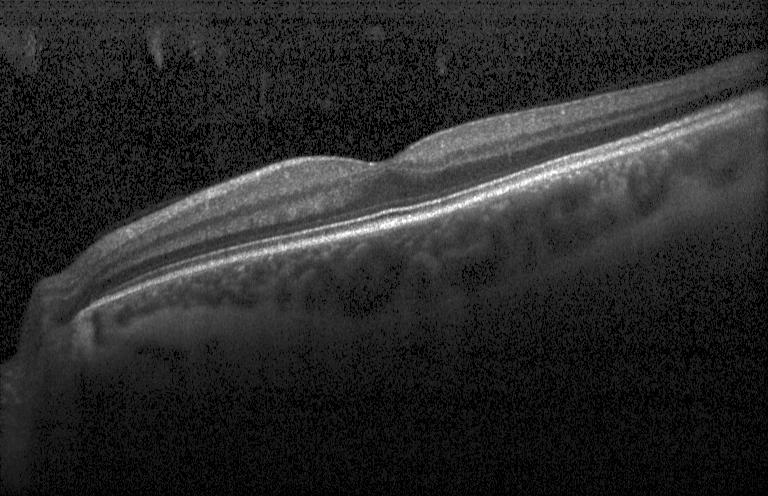
Dx: neither choroidal neovascularization, diabetic macular edema, nor drusen.